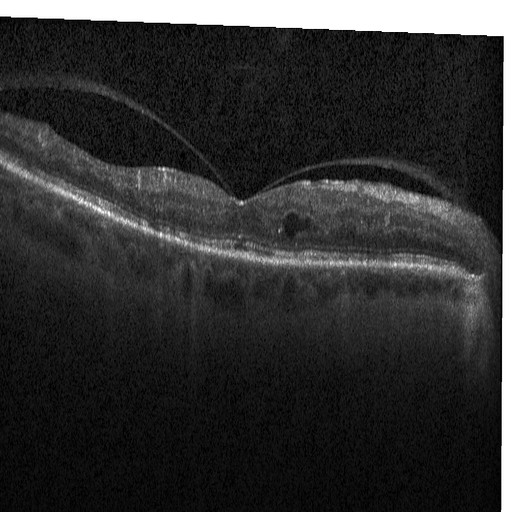
Acquired on a Heidelberg Spectralis, through the macula, optical coherence tomography scan
Impression: diabetic macular edema.